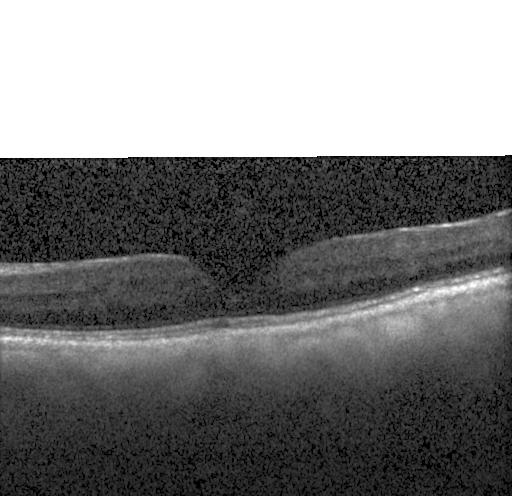 Retinal OCT cross-section · Heidelberg Spectralis OCT system · spectral-domain optical coherence tomography
OCT finding: neither choroidal neovascularization, diabetic macular edema, nor drusen.